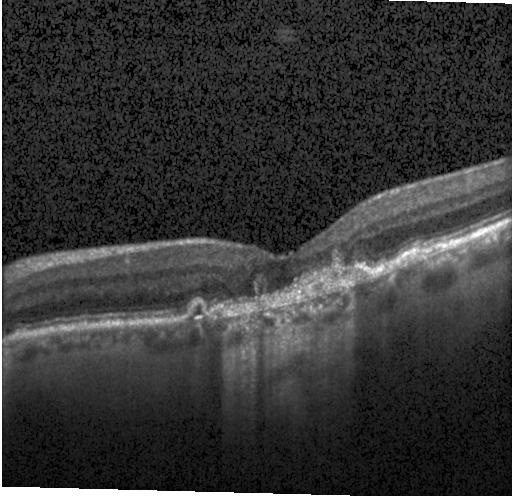 Choroidal neovascularization.